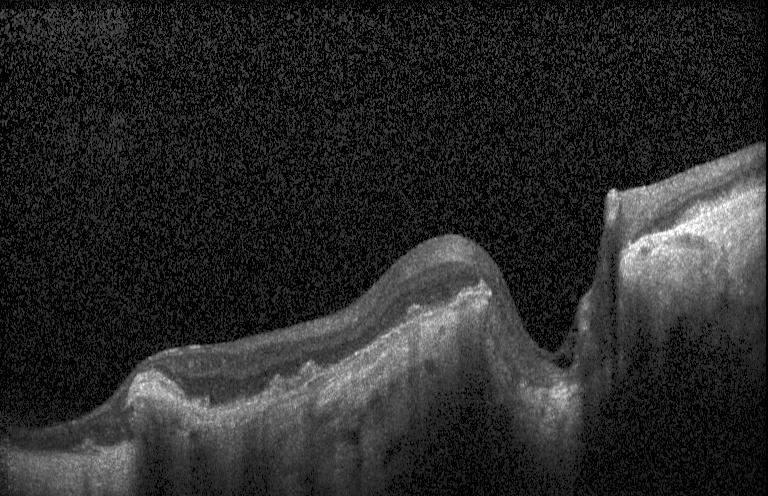
SD-OCT, optical coherence tomography B-scan — Assessment: a choroidal neovascular membrane.